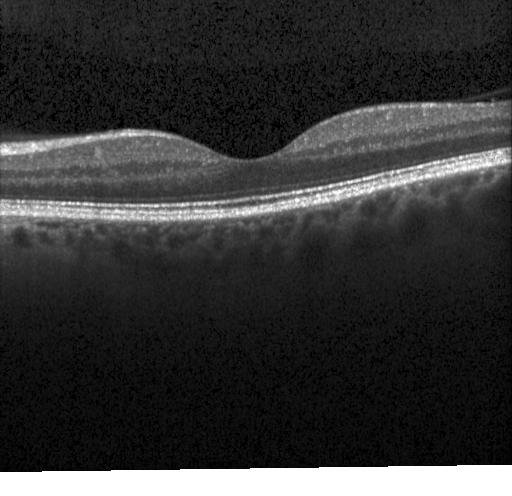 Retinal OCT B-scan. Spectral-domain OCT. Macular scan. Instrument: Heidelberg Spectralis
Impression: neither choroidal neovascularization, diabetic macular edema, nor drusen.